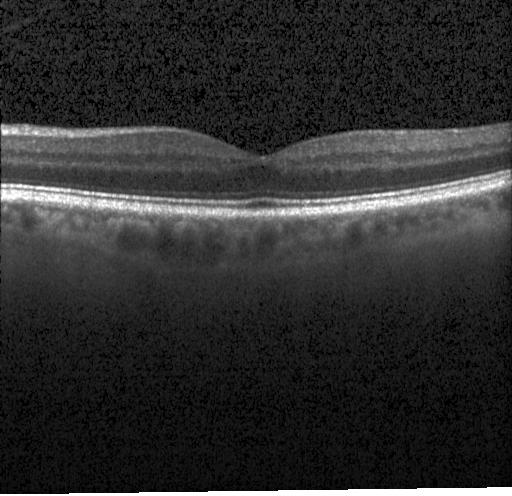
Retinal OCT B-scan. Acquired on a Heidelberg Spectralis. SD-OCT. Through the macula
Impression: no choroidal neovascularization, diabetic macular edema, or drusen.